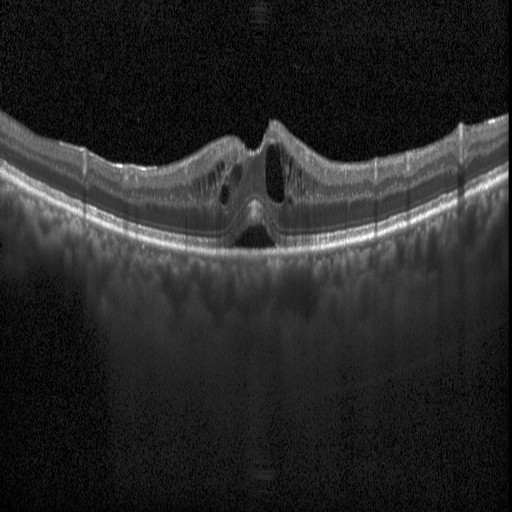

Macular OCT demonstrating diabetic macular edema.